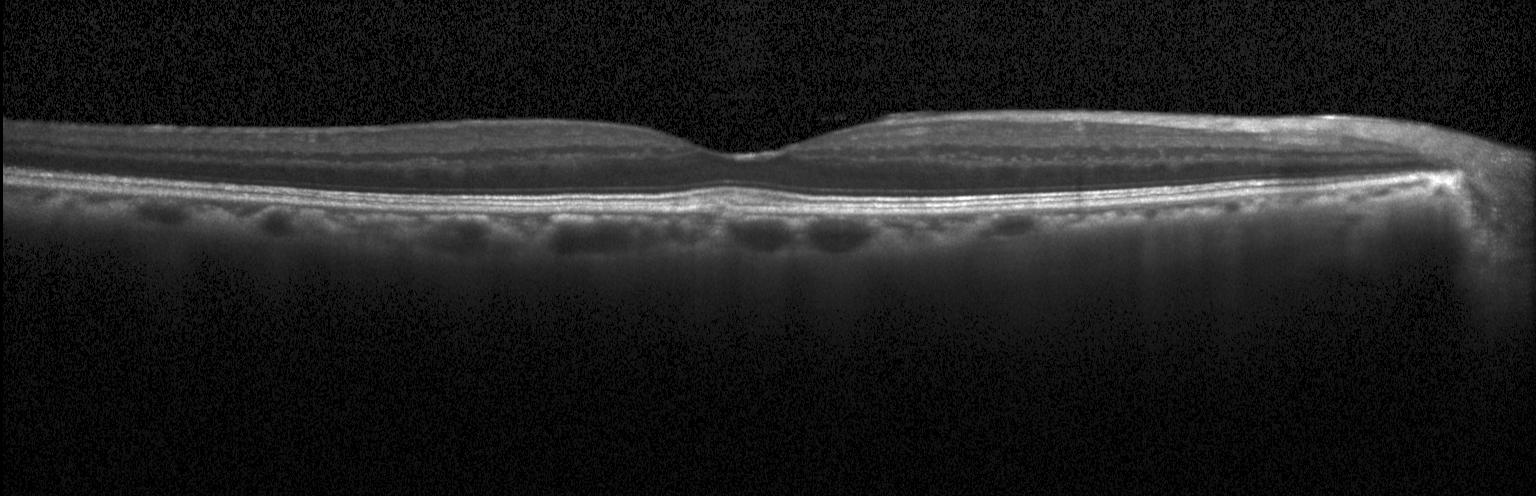
Dx: no evidence of choroidal neovascularization, diabetic macular edema, or drusen.